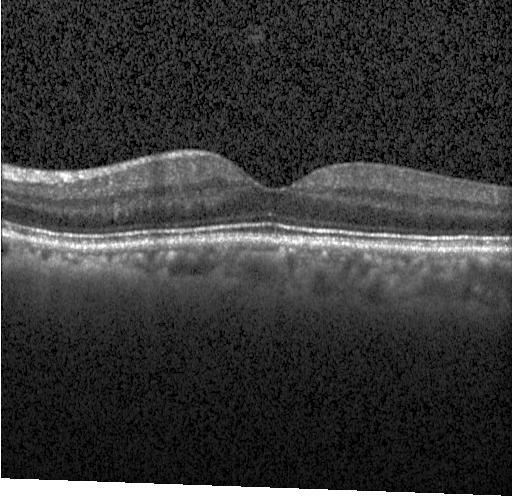
OCT finding: no CNV, no DME, and no drusen.